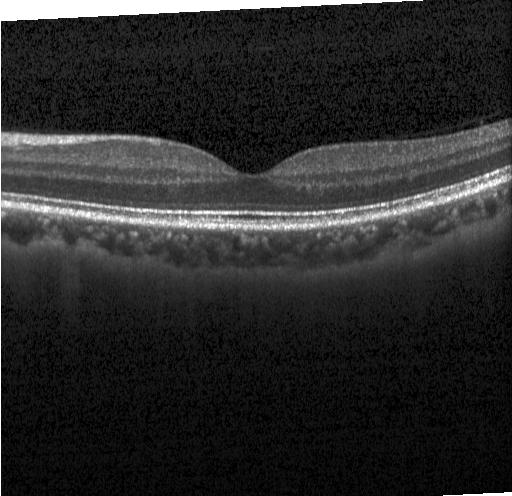 Macular OCT: neither CNV, DME, nor drusen.